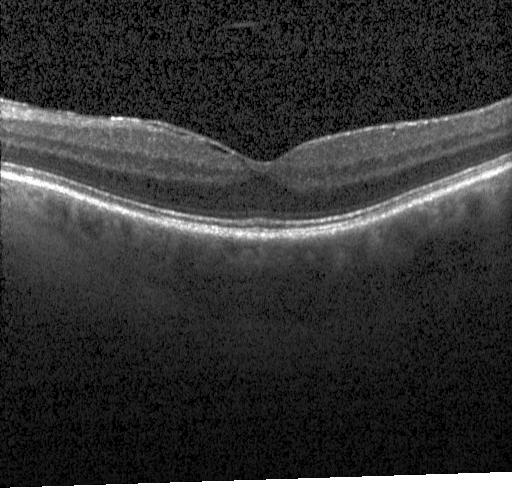 Retinal OCT B-scan.
Diagnosis: neither choroidal neovascularization, diabetic macular edema, nor drusen.